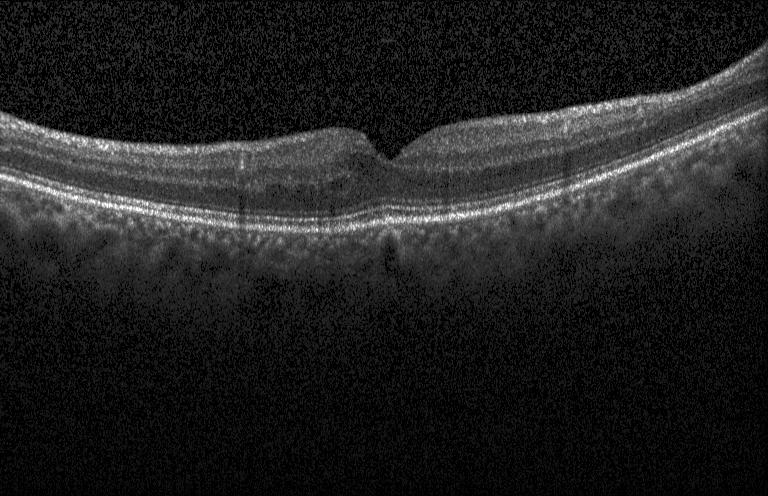
Retinal OCT cross-section, SD-OCT, through the macula — This B-scan demonstrates DME.